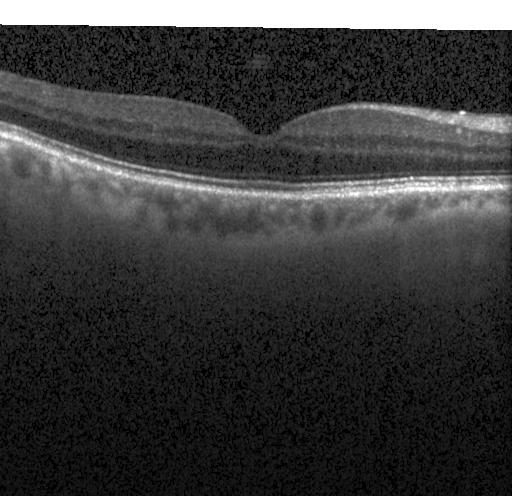

Spectral-domain OCT B-scan: neither choroidal neovascularization, diabetic macular edema, nor drusen.